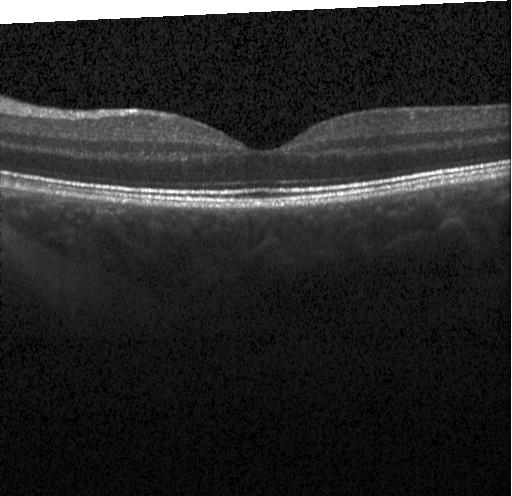 Macular OCT: no choroidal neovascularization, diabetic macular edema, or drusen.